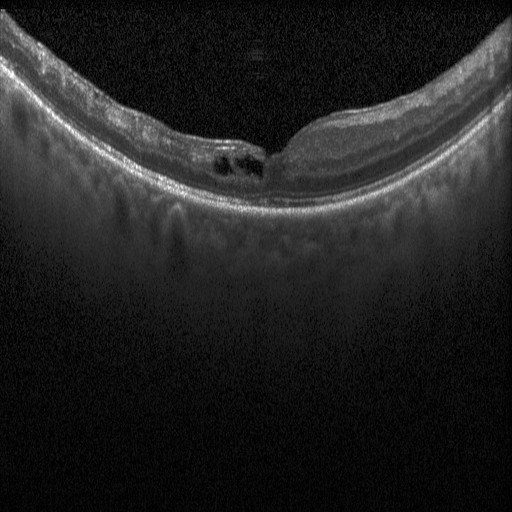

Finding: diabetic macular edema (DME).